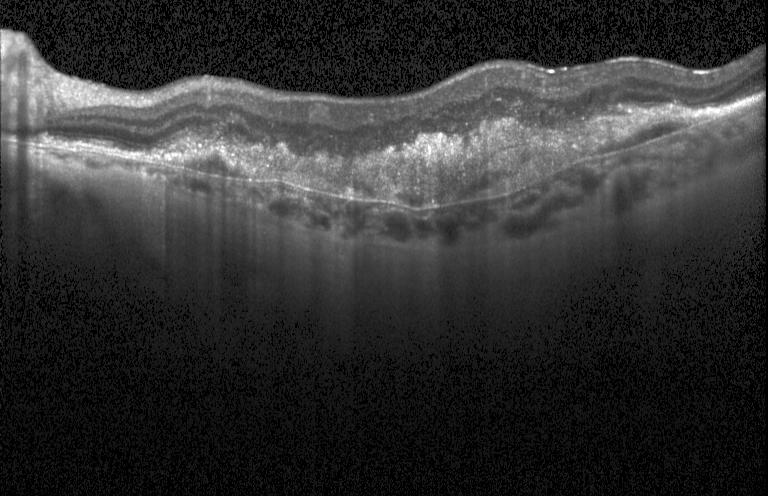 OCT finding: choroidal neovascularization (CNV).